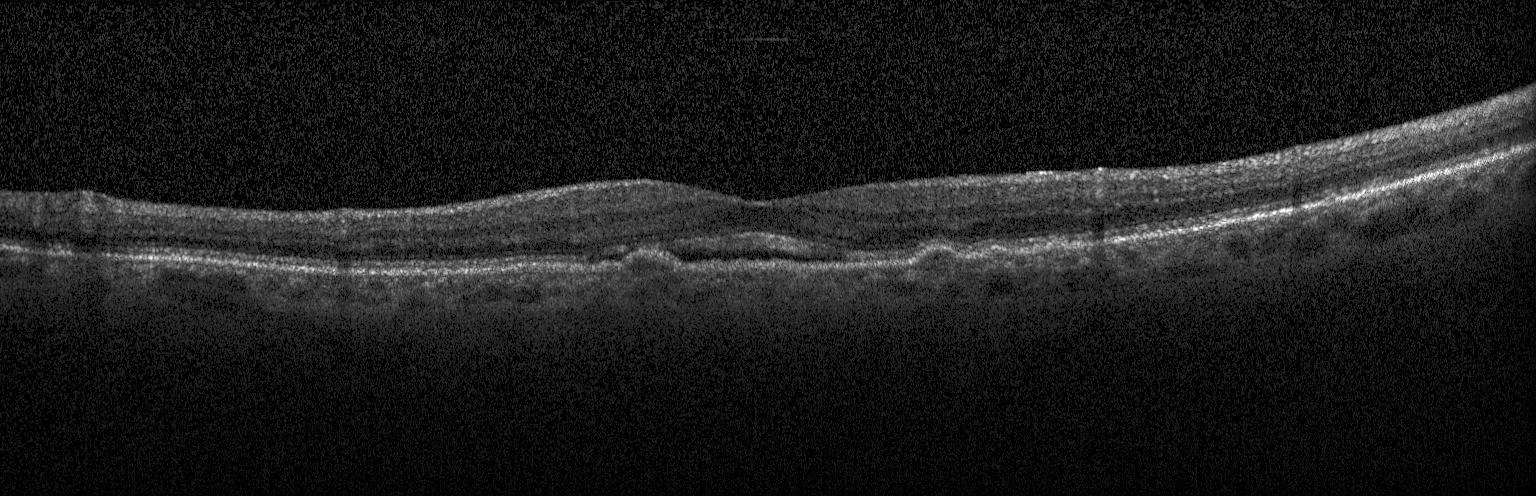 Diagnosis: CNV.